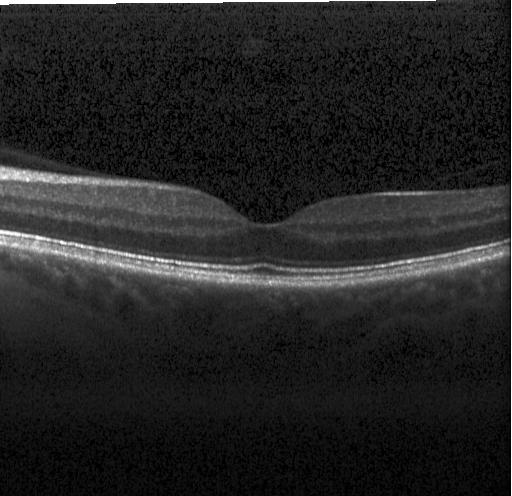 Spectral-domain OCT B-scan: no choroidal neovascularization, diabetic macular edema, or drusen.